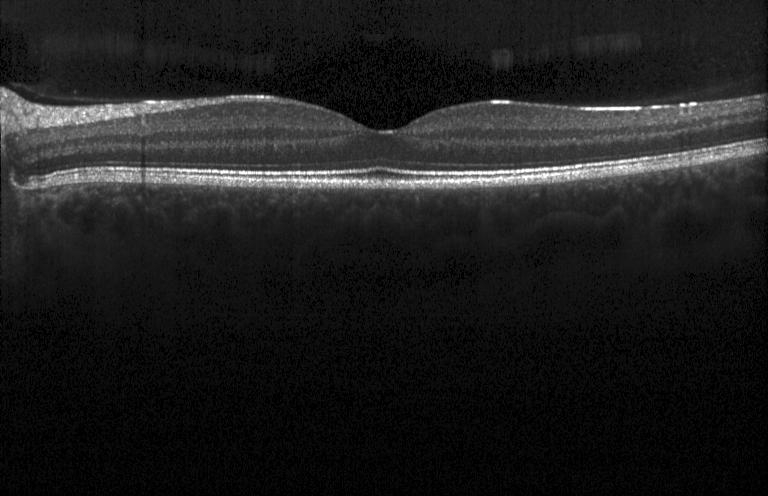 Horizontal scan through the fovea. Heidelberg Spectralis. Spectral-domain optical coherence tomography. Retinal OCT cross-section — The scan shows no choroidal neovascularization, diabetic macular edema, or drusen.